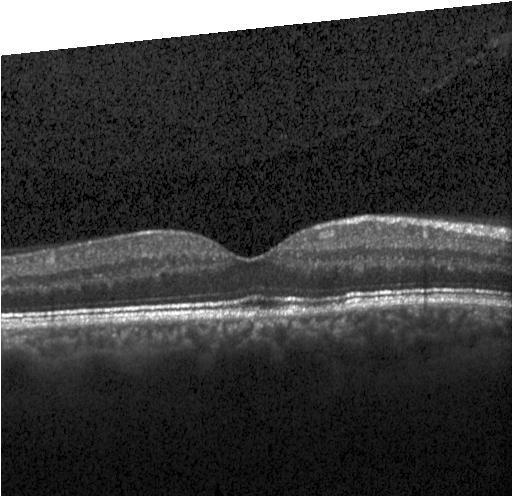
No choroidal neovascularization, no diabetic macular edema, and no drusen.